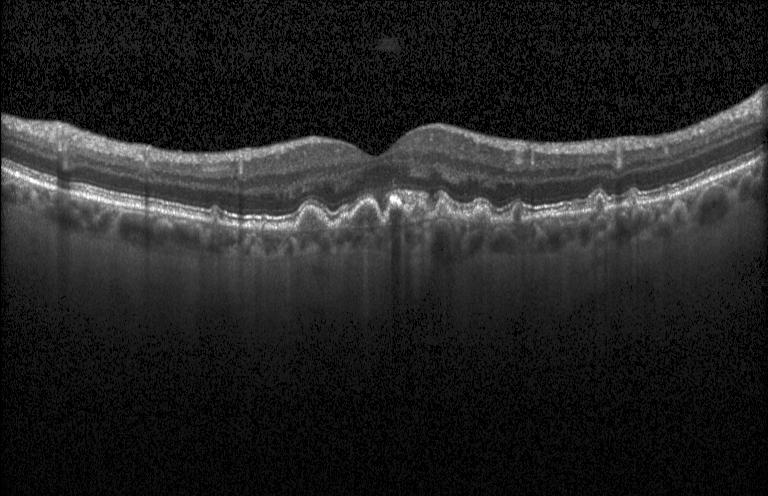 Spectral-domain OCT B-scan: sub-RPE drusenoid deposits.